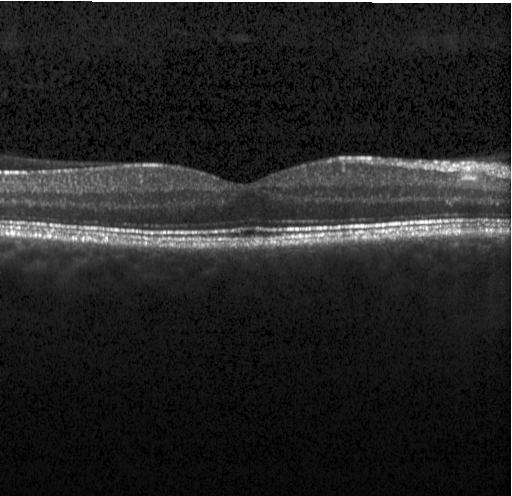

Impression: no choroidal neovascularization, no diabetic macular edema, and no drusen.